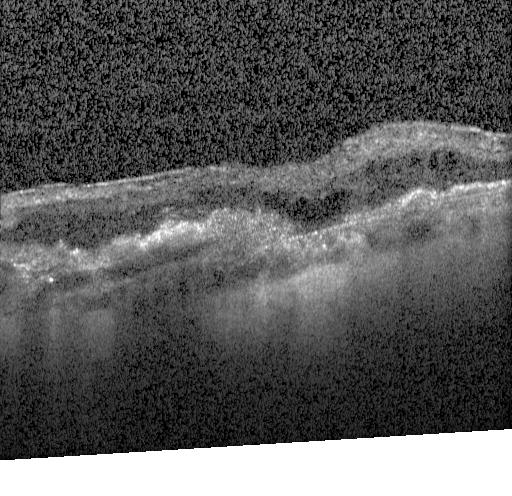
Spectral-domain OCT B-scan: a choroidal neovascular membrane.